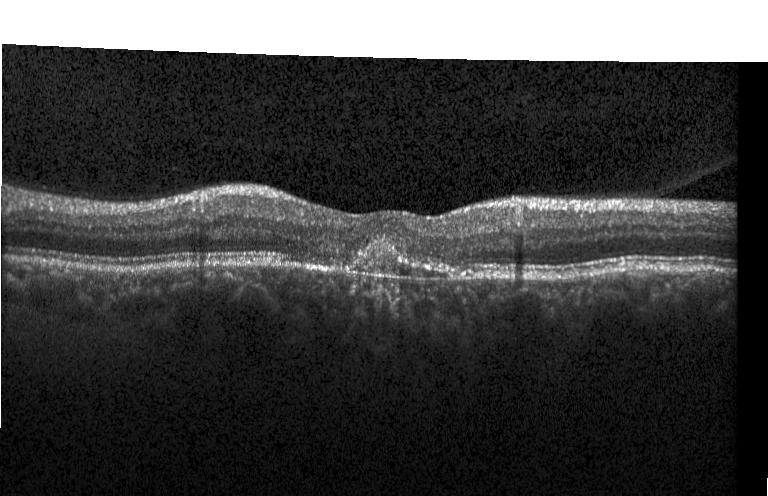
OCT finding: a choroidal neovascular membrane.